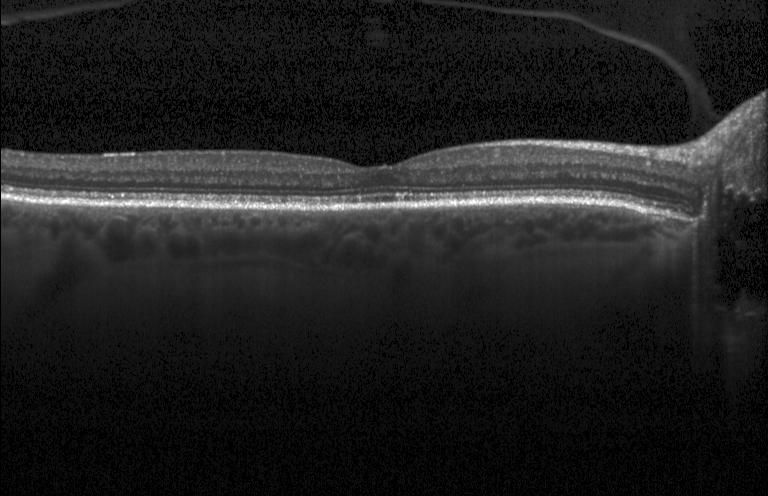
OCT B-scan, fovea-centered. Impression: no choroidal neovascularization, no diabetic macular edema, and no drusen.